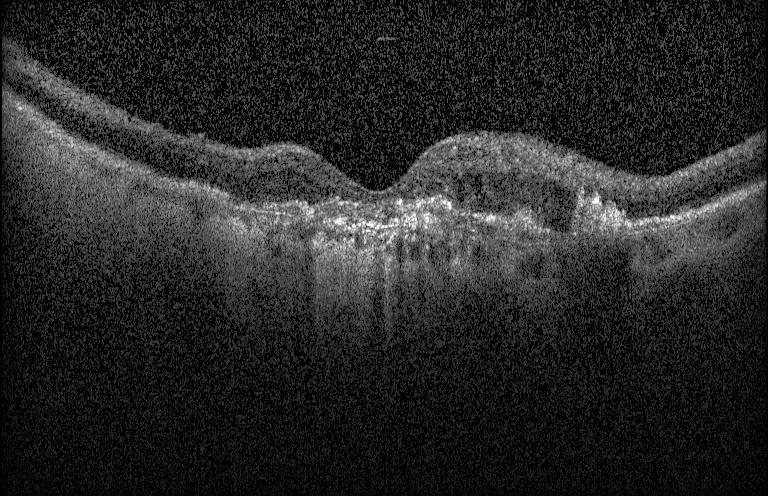

Macular OCT demonstrating choroidal neovascularization.